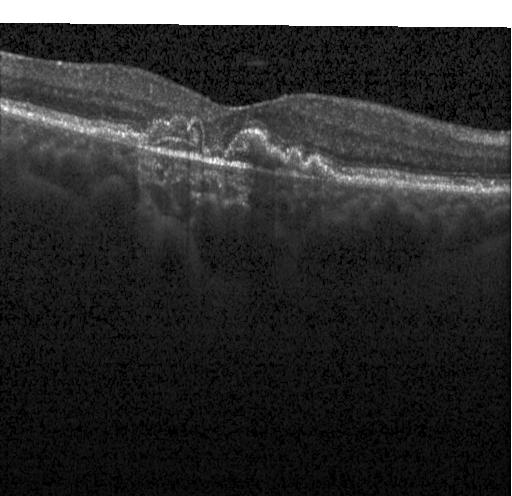 Spectral-domain optical coherence tomography. Macular scan. Heidelberg Spectralis. Optical coherence tomography B-scan. Dx: choroidal neovascularization (CNV).